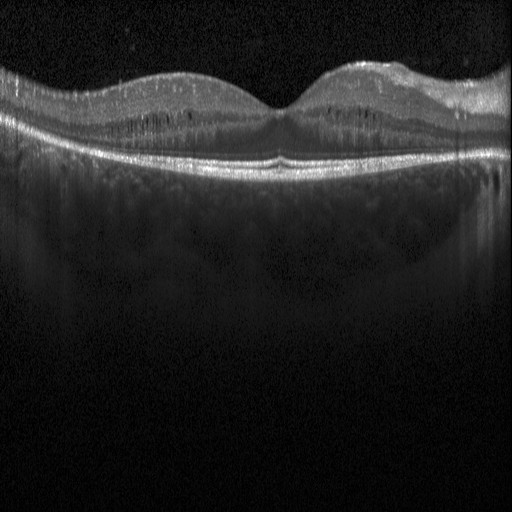
Retinal OCT cross-section showing diabetic macular edema (DME).